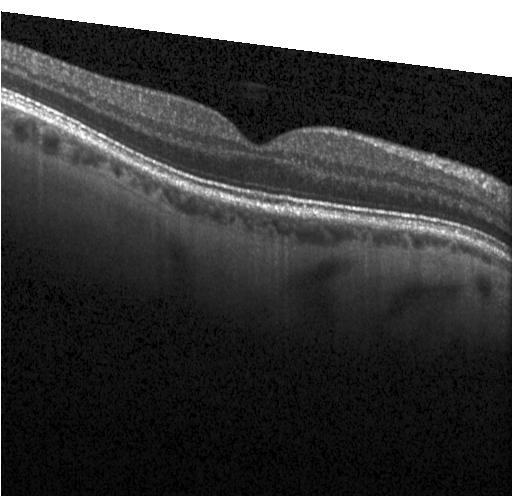 Diagnosis: no evidence of choroidal neovascularization, diabetic macular edema, or drusen.